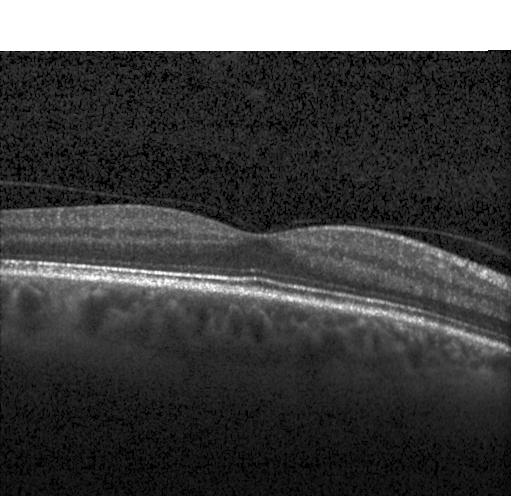
Horizontal scan through the fovea; retinal OCT cross-section; spectral-domain optical coherence tomography.
Diagnosis: neither CNV, DME, nor drusen.